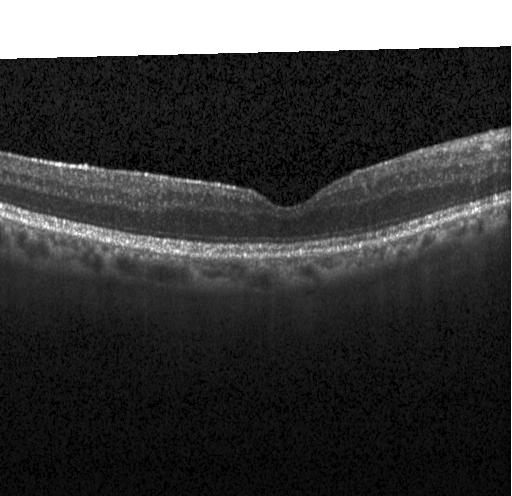

Retinal OCT cross-section.
Impression: no CNV, DME, or drusen.